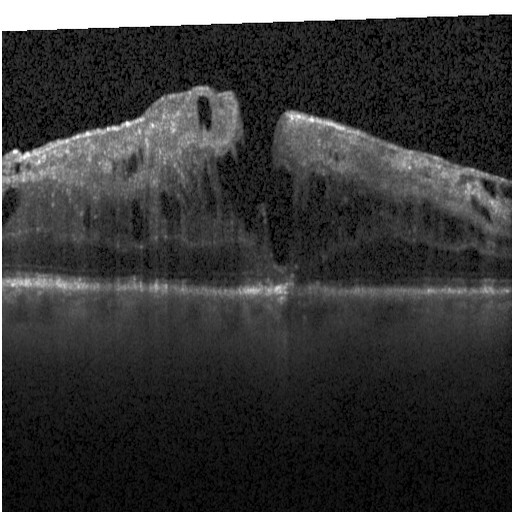

Macular scan; OCT line scan
Finding: DME.